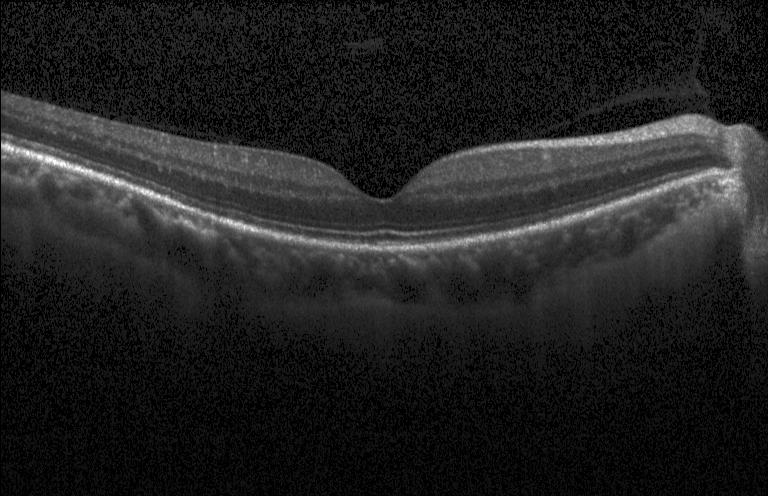

SD-OCT, Heidelberg Spectralis OCT system, retinal OCT B-scan. OCT finding: no choroidal neovascularization, no diabetic macular edema, and no drusen.